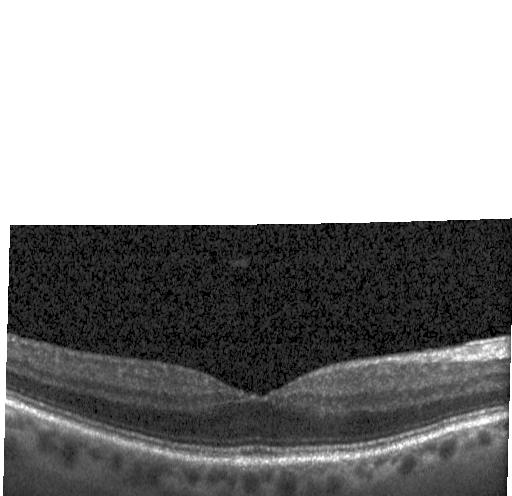 Through the macula; retinal OCT B-scan; spectral-domain optical coherence tomography; instrument: Heidelberg Spectralis.
Finding: no choroidal neovascularization, diabetic macular edema, or drusen.